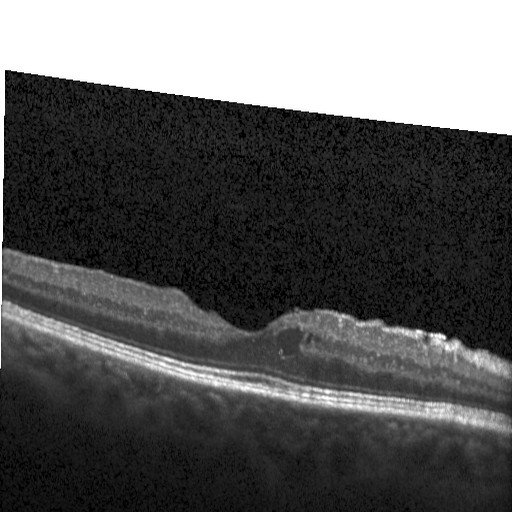

Optical coherence tomography B-scan · spectral-domain OCT · horizontal scan through the fovea · acquired on a Heidelberg Spectralis
Finding: diabetic macular edema.